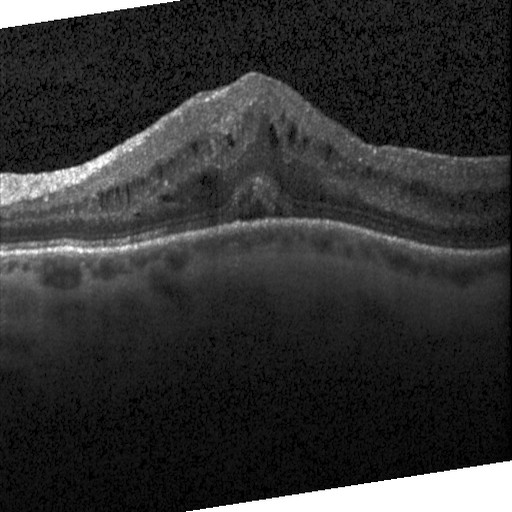
OCT line scan, macular scan
Diagnosis: DME.